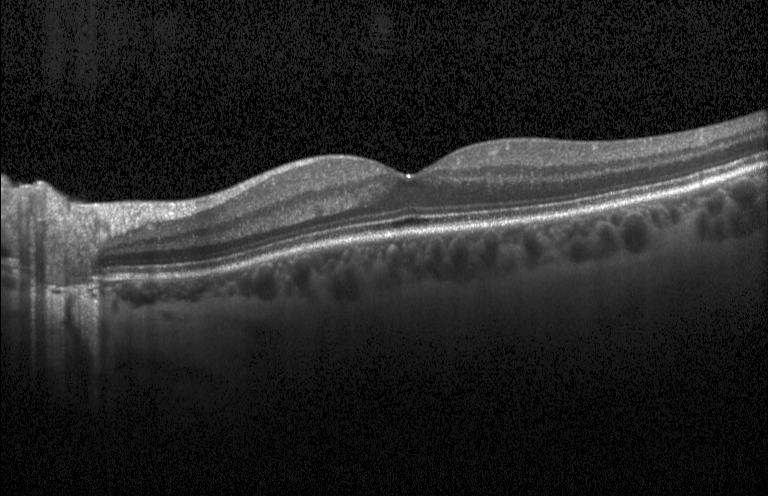
Optical coherence tomography B-scan; spectral-domain OCT. The scan shows no evidence of choroidal neovascularization, diabetic macular edema, or drusen.